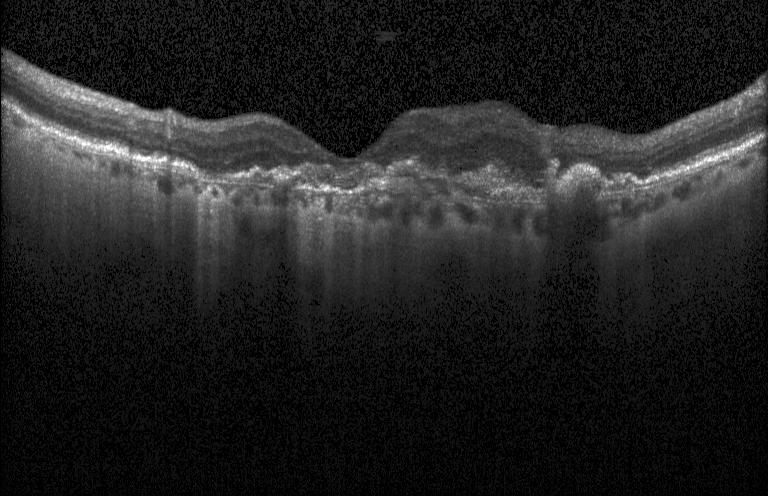

Optical coherence tomography scan
The scan shows a choroidal neovascular membrane.